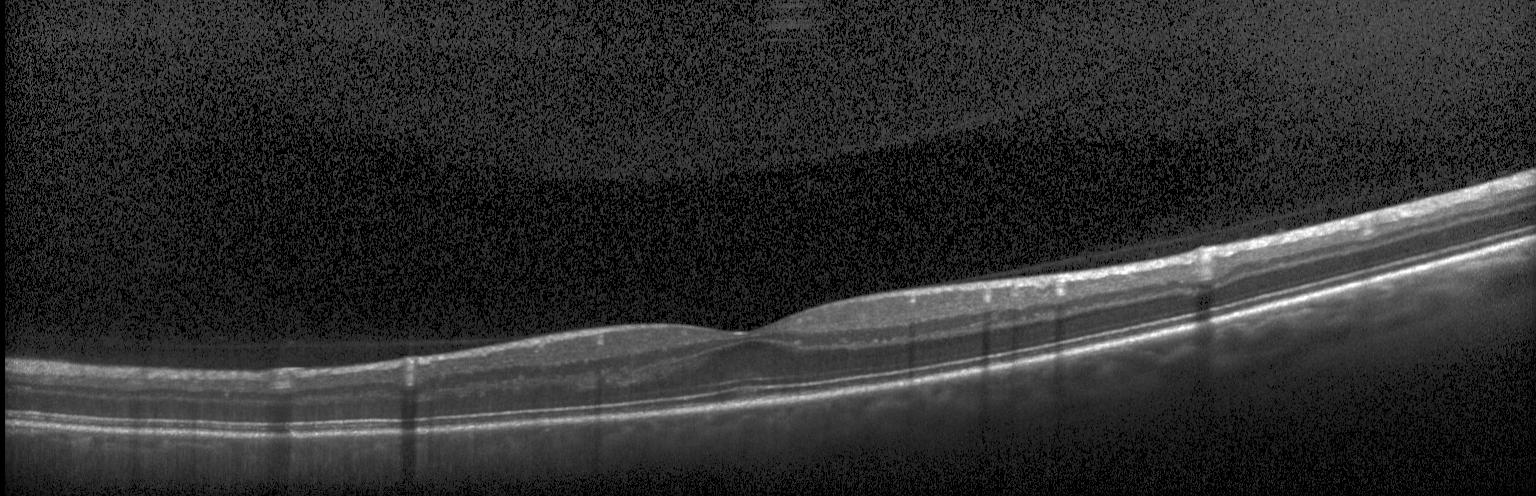

Optical coherence tomography B-scan. Through the macula. Spectral-domain optical coherence tomography. Instrument: Heidelberg Spectralis.
This B-scan demonstrates no CNV, DME, or drusen.